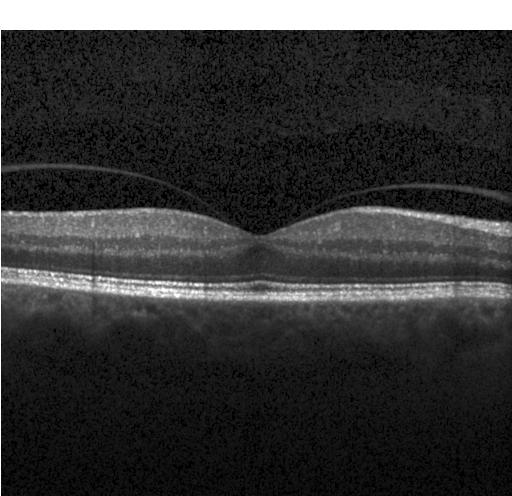

Optical coherence tomography B-scan.
Diagnosis: no choroidal neovascularization, no diabetic macular edema, and no drusen.